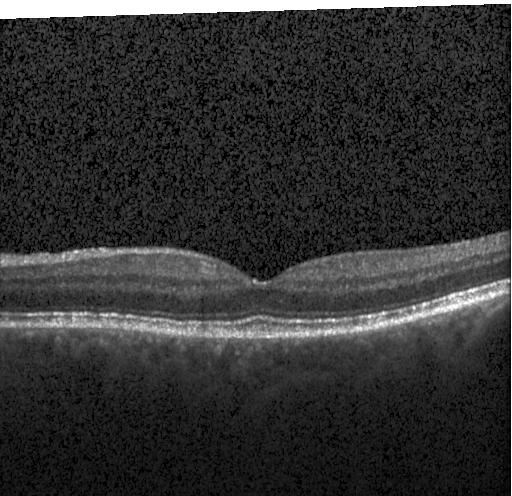

Optical coherence tomography scan · Heidelberg Spectralis
No choroidal neovascularization, diabetic macular edema, or drusen.